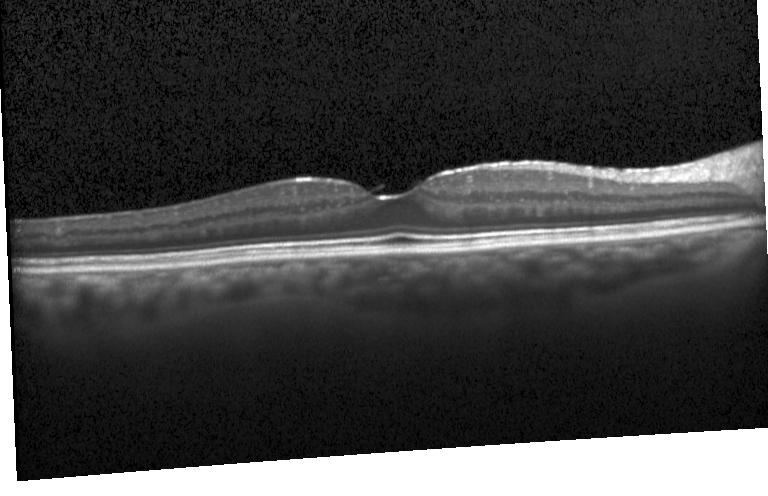

Optical coherence tomography scan
OCT finding: no evidence of CNV, DME, or drusen.